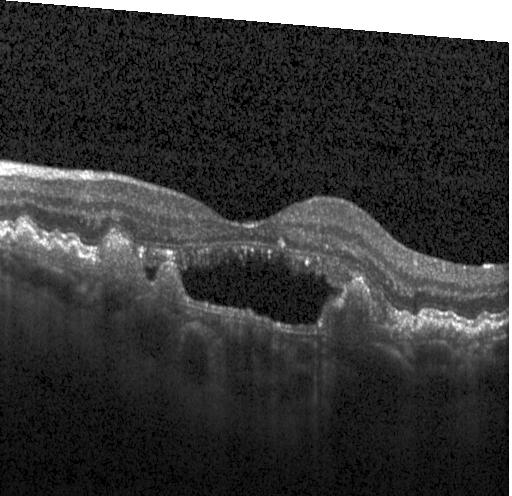
Through the macula, optical coherence tomography B-scan, Heidelberg Spectralis
A choroidal neovascular membrane.